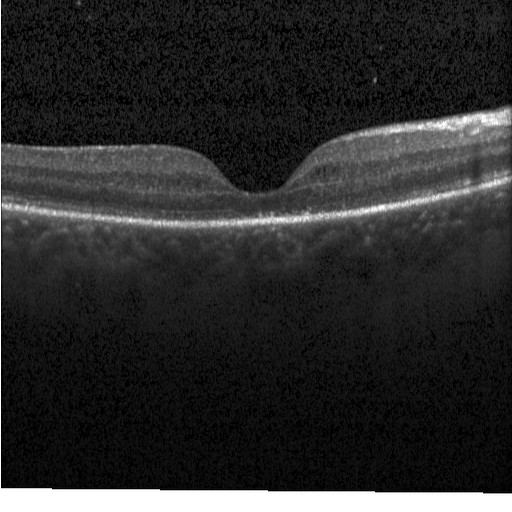

Impression: diabetic macular edema.